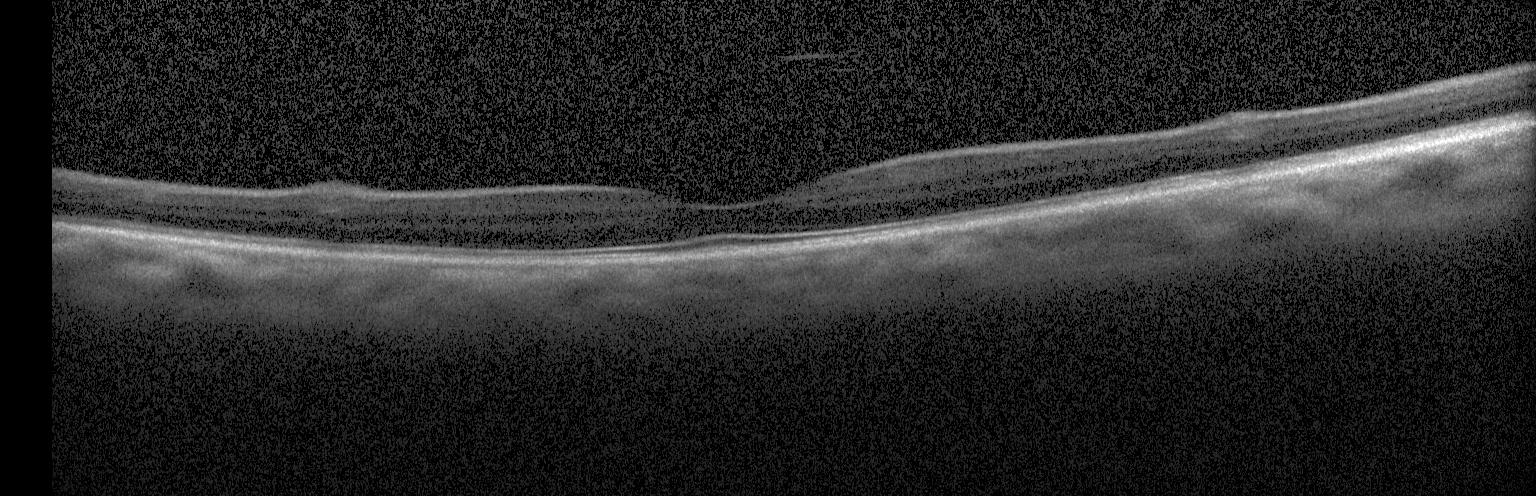
Retinal OCT B-scan. Diagnosis: neither choroidal neovascularization, diabetic macular edema, nor drusen.